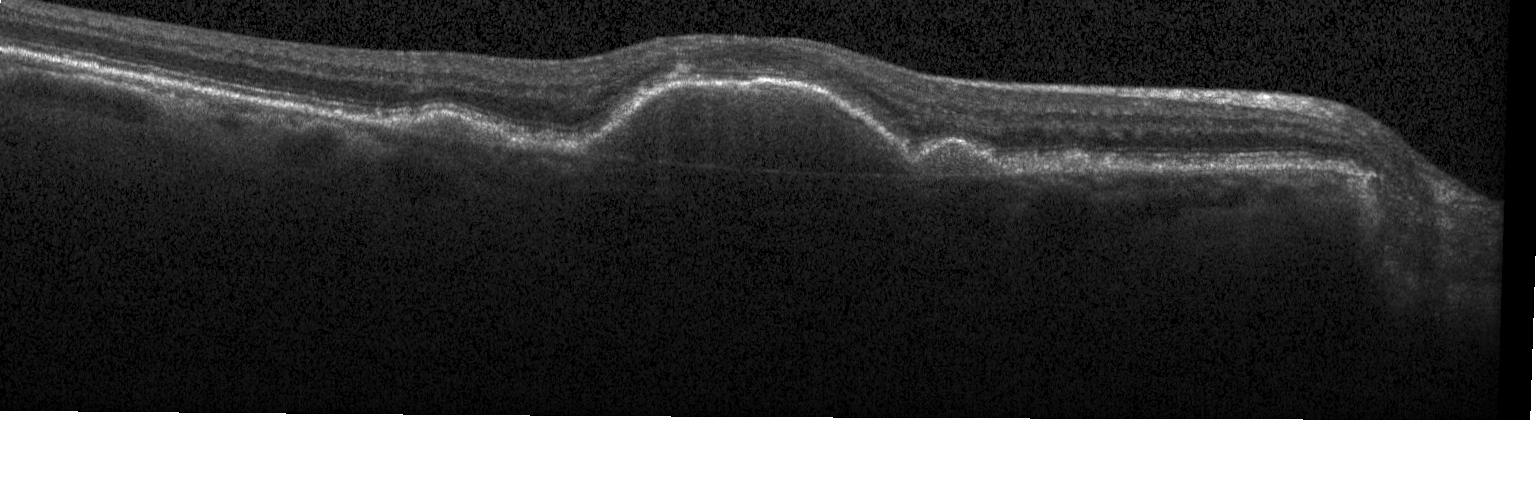

OCT line scan · spectral-domain optical coherence tomography — Diagnosis: a choroidal neovascular membrane.